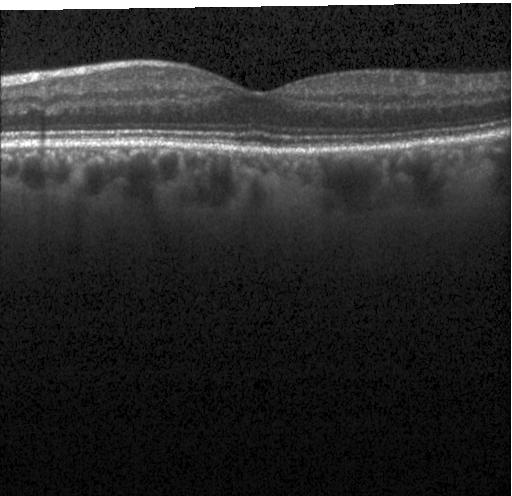
Dx: neither choroidal neovascularization, diabetic macular edema, nor drusen.